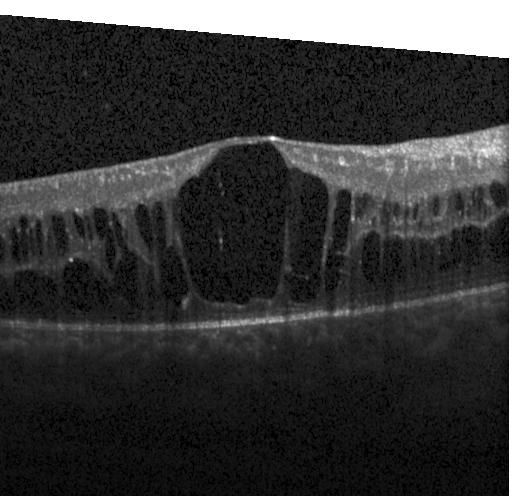 Macular OCT: diabetic macular edema.